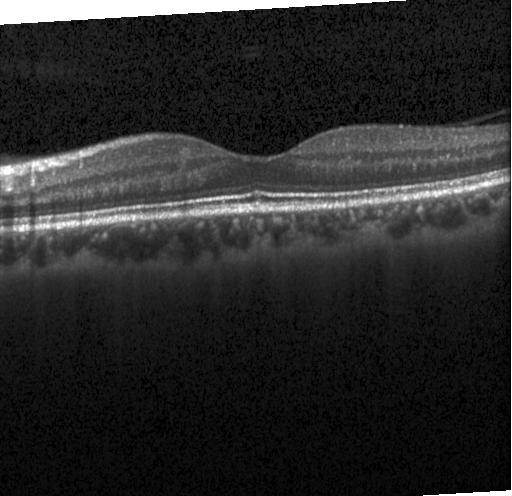
OCT B-scan showing no evidence of choroidal neovascularization, diabetic macular edema, or drusen.